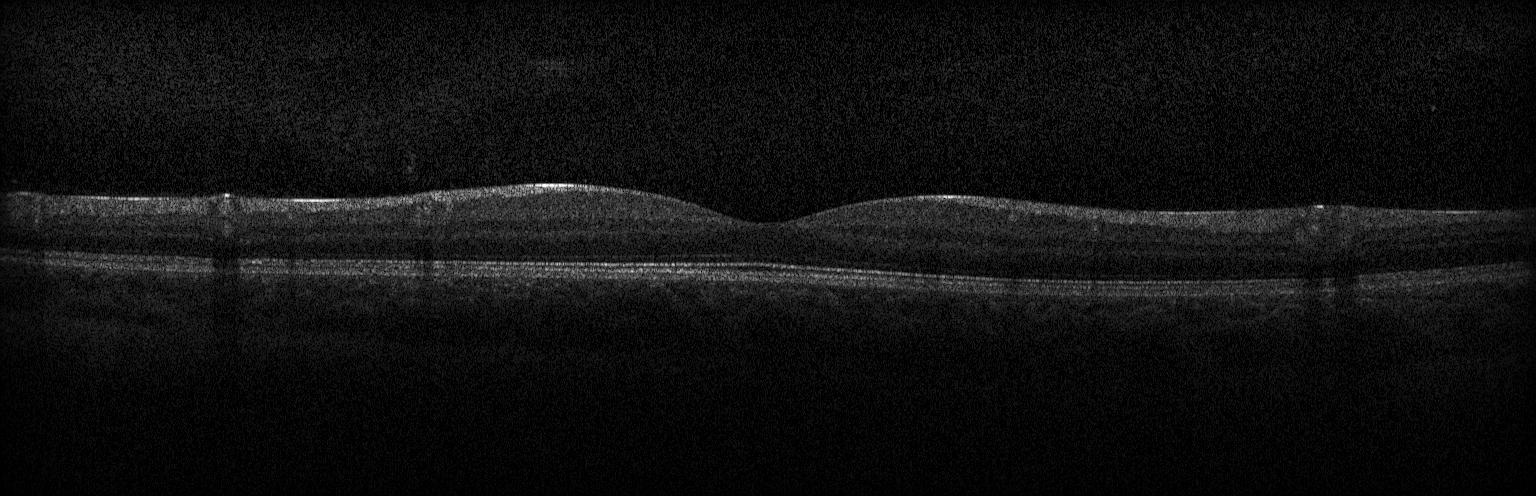

Optical coherence tomography scan.
This B-scan demonstrates no choroidal neovascularization, no diabetic macular edema, and no drusen.